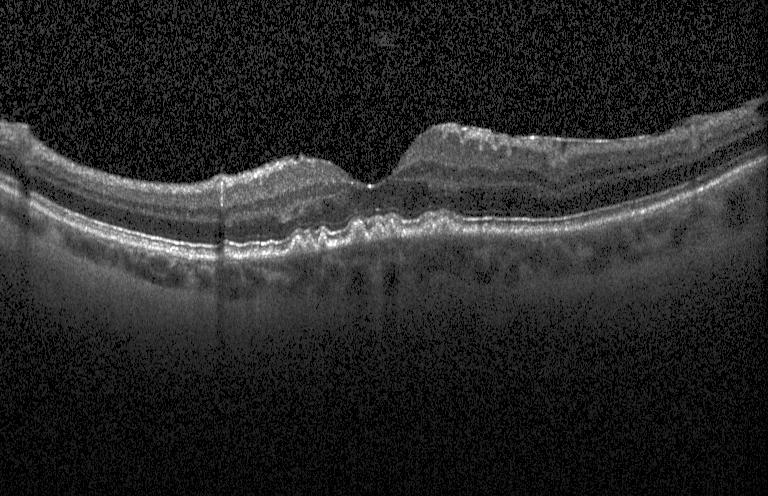

Retinal OCT cross-section. Heidelberg Spectralis OCT system — The scan shows sub-RPE drusenoid deposits.